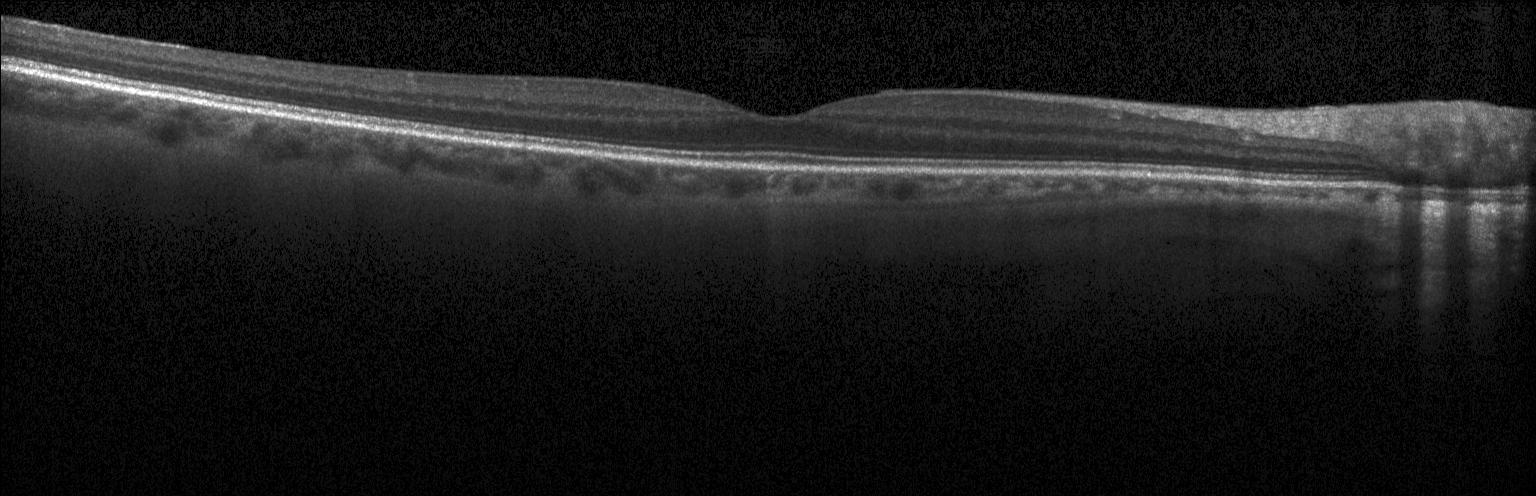

The scan shows no CNV, DME, or drusen.